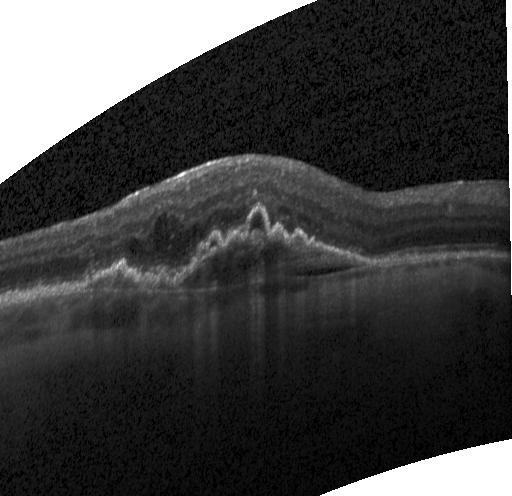 Retinal OCT cross-section — Choroidal neovascularization (CNV).